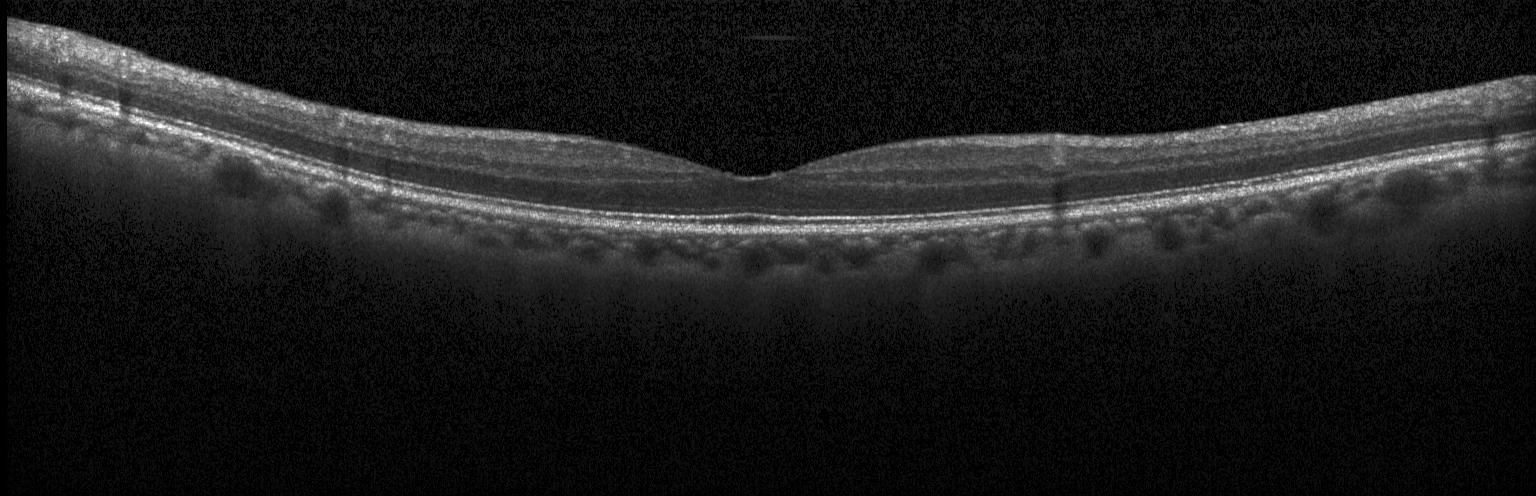 Retinal OCT cross-section · spectral-domain OCT — Assessment: no choroidal neovascularization, no diabetic macular edema, and no drusen.